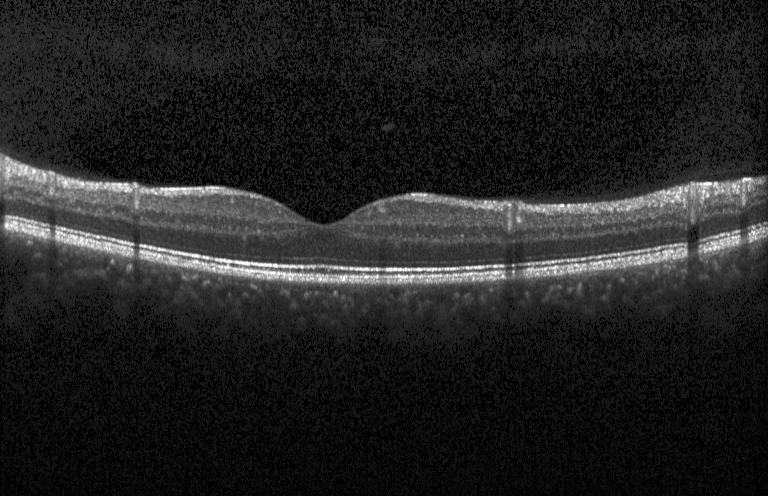 SD-OCT; acquired on a Heidelberg Spectralis; horizontal scan through the fovea; optical coherence tomography B-scan
This B-scan demonstrates no evidence of choroidal neovascularization, diabetic macular edema, or drusen.